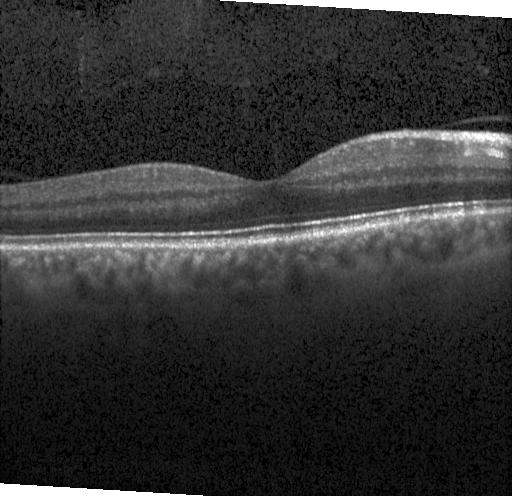 Macular OCT: neither CNV, DME, nor drusen.